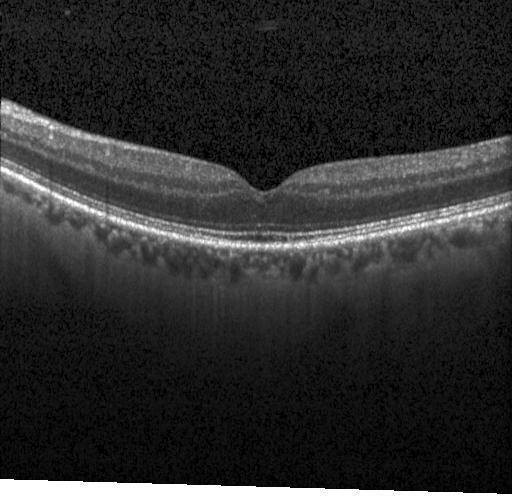 Retinal OCT B-scan.
Finding: no evidence of CNV, DME, or drusen.